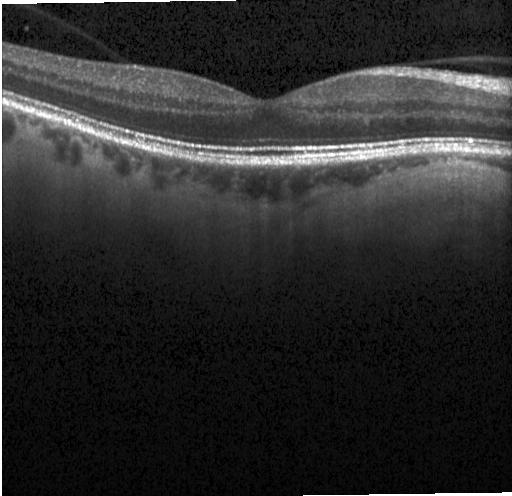
OCT B-scan.
The scan shows no choroidal neovascularization, diabetic macular edema, or drusen.